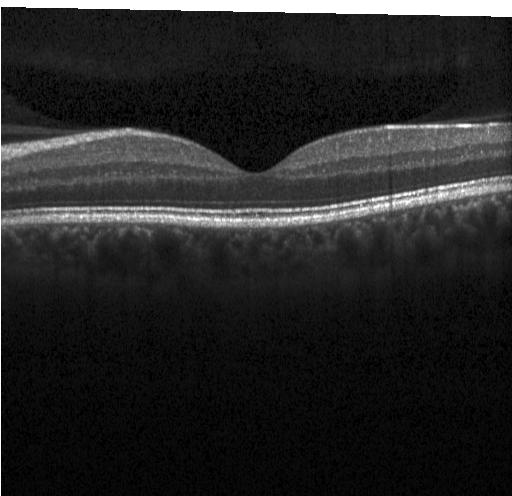
Spectral-domain optical coherence tomography; optical coherence tomography scan; acquired on a Heidelberg Spectralis; fovea-centered
Diagnosis: no choroidal neovascularization, diabetic macular edema, or drusen.